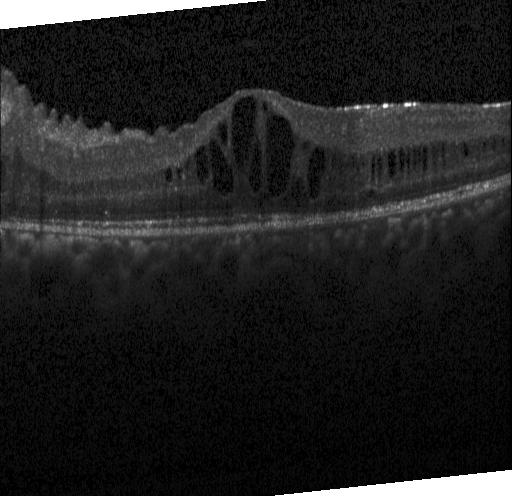

Macular OCT: diabetic macular edema (DME).